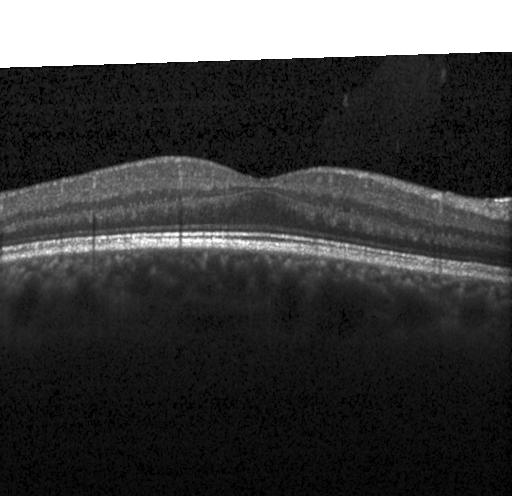
The scan shows no evidence of choroidal neovascularization, diabetic macular edema, or drusen.